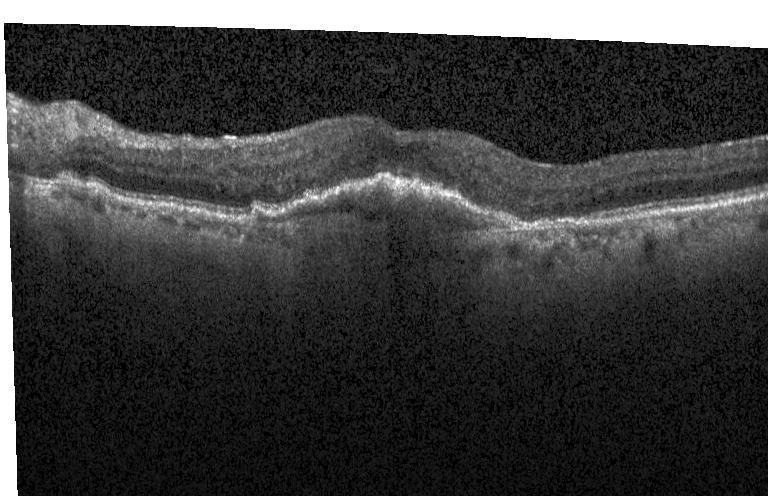 Spectral-domain OCT · retinal OCT cross-section · Heidelberg Spectralis — OCT finding: a choroidal neovascular membrane.